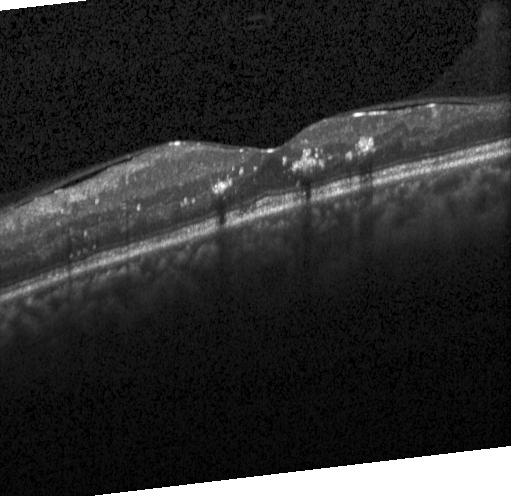 Impression: DME.